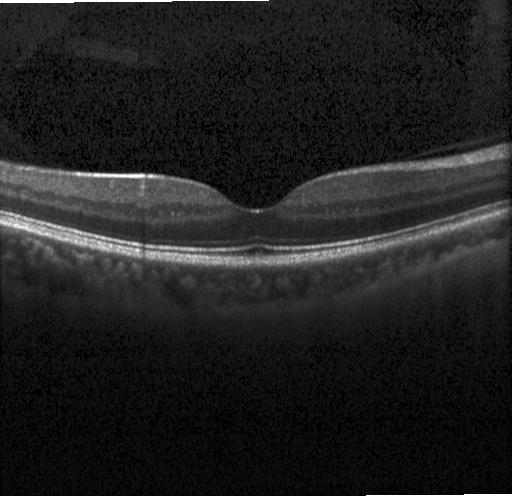

Spectral-domain optical coherence tomography, Heidelberg Spectralis OCT system, OCT line scan — Impression: neither choroidal neovascularization, diabetic macular edema, nor drusen.